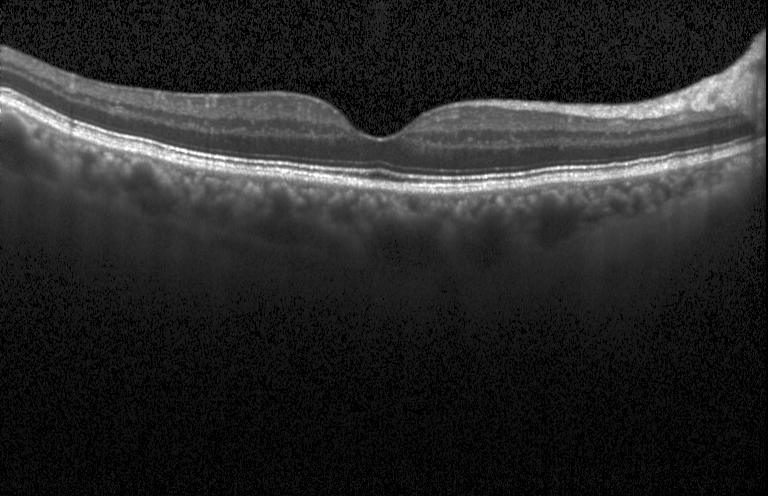

Retinal OCT cross-section showing no evidence of choroidal neovascularization, diabetic macular edema, or drusen.